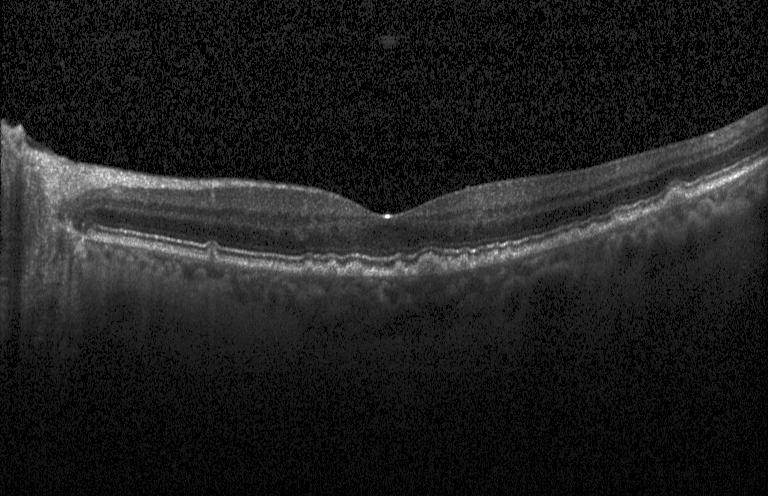

Optical coherence tomography scan.
Dx: multiple drusen.